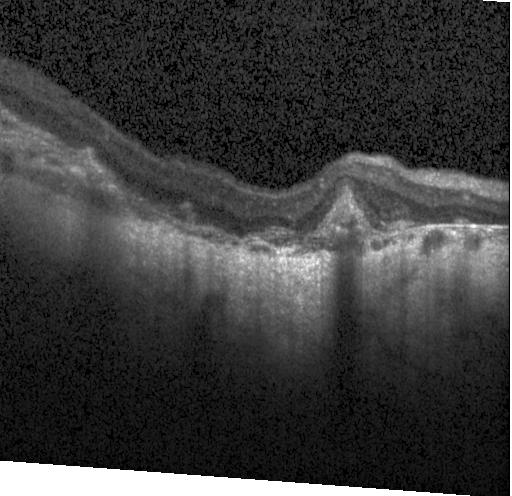
Optical coherence tomography scan; spectral-domain OCT. Finding: choroidal neovascularization.